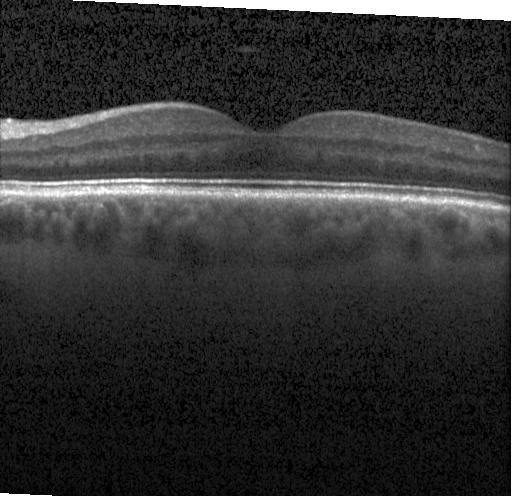

OCT B-scan · Heidelberg Spectralis OCT system
Diagnosis: no CNV, DME, or drusen.